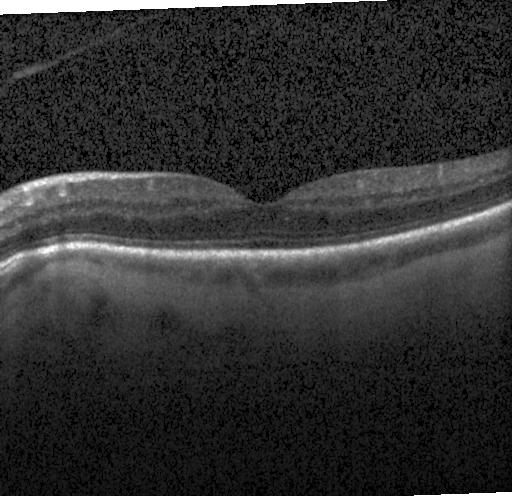
This B-scan demonstrates no CNV, DME, or drusen.